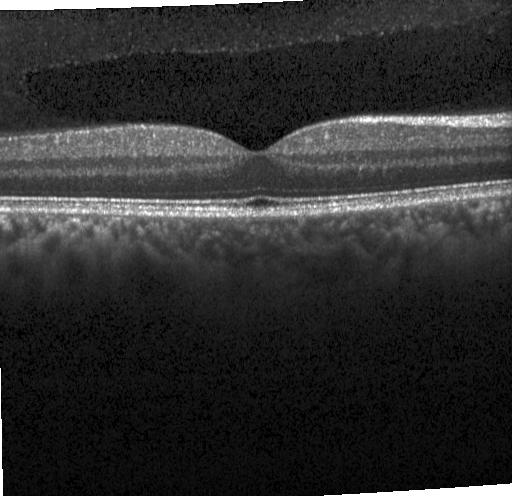

Retinal OCT B-scan · acquired on a Heidelberg Spectralis · fovea-centered.
No CNV, no DME, and no drusen.